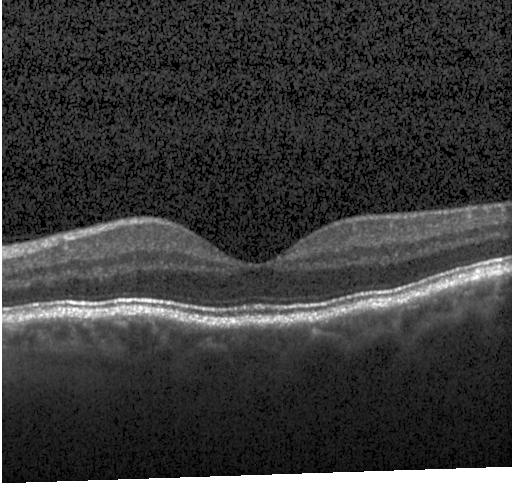 OCT line scan. Diagnosis: no choroidal neovascularization, no diabetic macular edema, and no drusen.